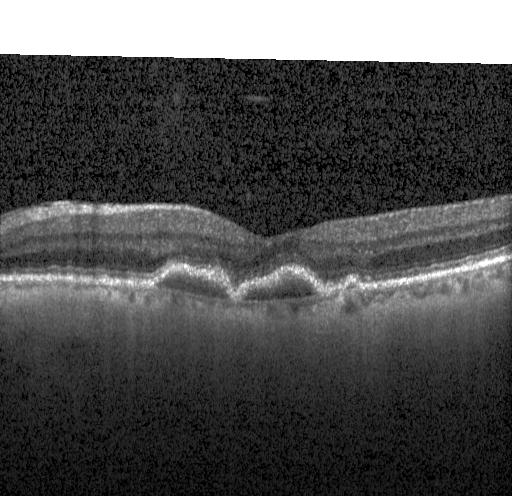

OCT line scan. Heidelberg Spectralis OCT system. SD-OCT — Dx: a choroidal neovascular membrane.